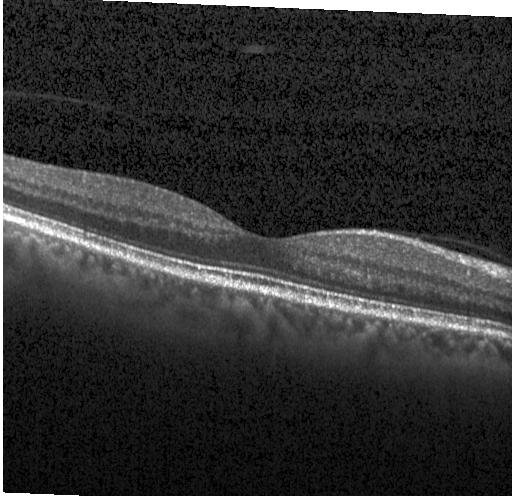

Diagnosis: no CNV, DME, or drusen.